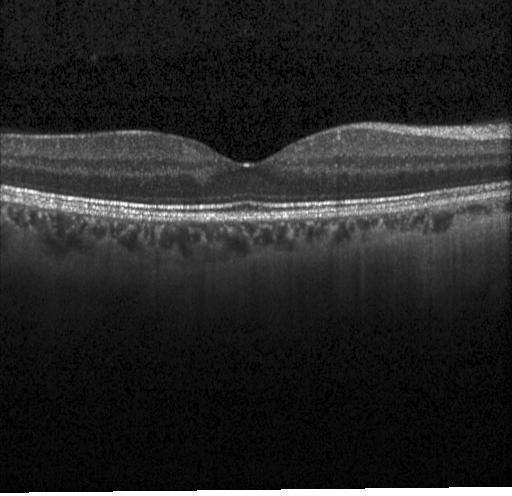
OCT B-scan showing no choroidal neovascularization, no diabetic macular edema, and no drusen.